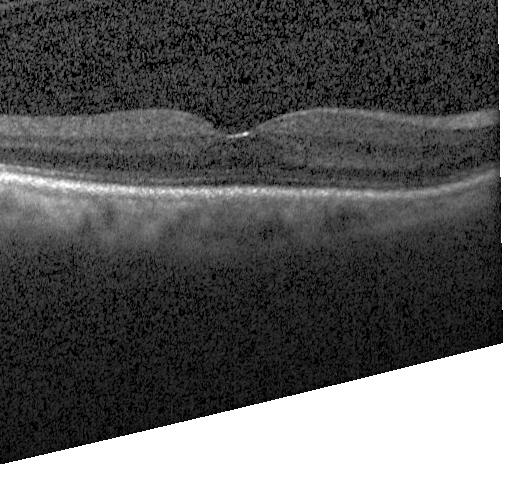
OCT B-scan
This B-scan demonstrates no evidence of CNV, DME, or drusen.